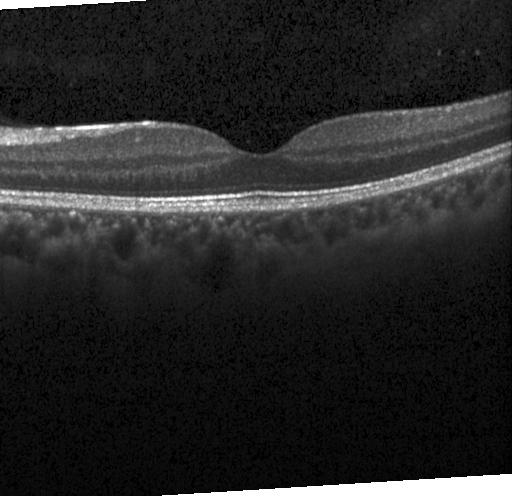

Impression: no evidence of choroidal neovascularization, diabetic macular edema, or drusen.